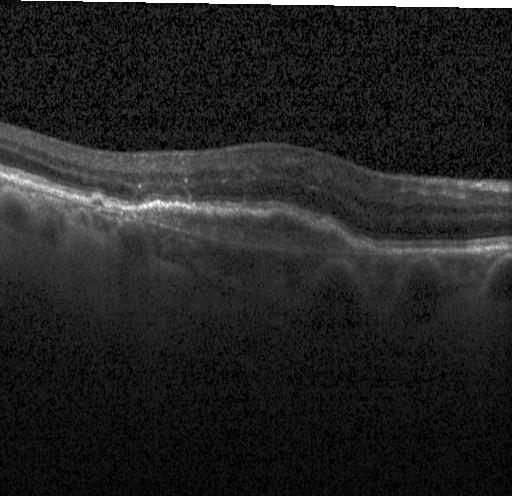
Diagnosis: a choroidal neovascular membrane.